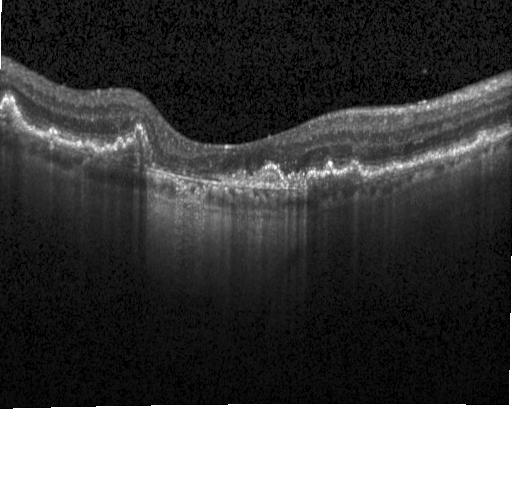

Diagnosis: a choroidal neovascular membrane.